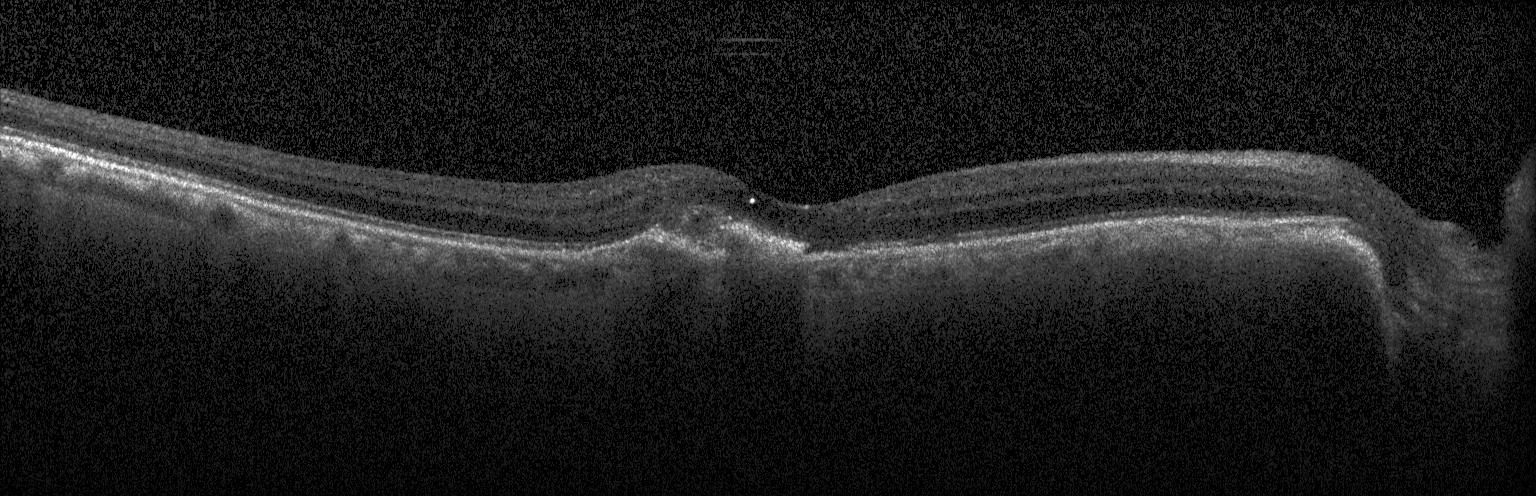

Optical coherence tomography scan; Heidelberg Spectralis. A choroidal neovascular membrane.